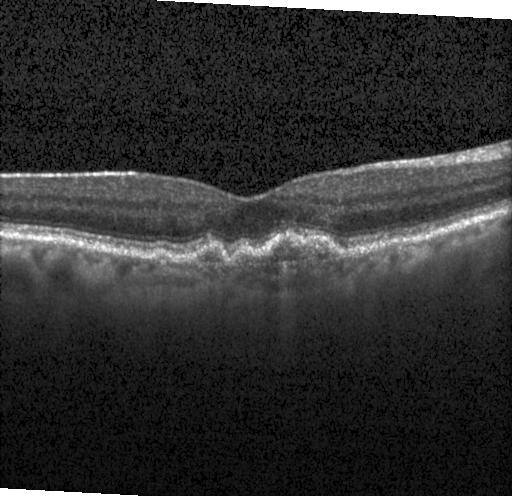

Retinal OCT cross-section · spectral-domain optical coherence tomography. Finding: a choroidal neovascular membrane.